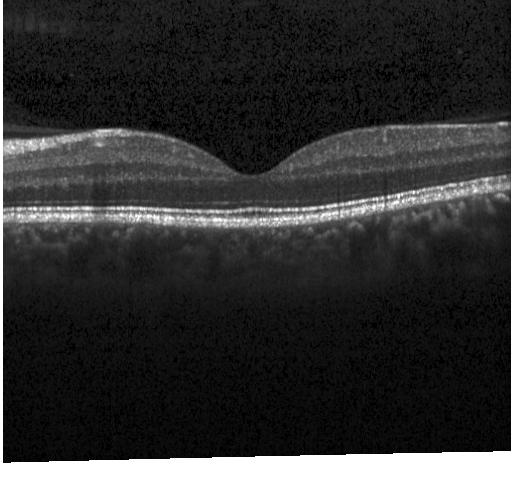

SD-OCT; centered on the fovea; OCT B-scan
The scan shows no CNV, no DME, and no drusen.